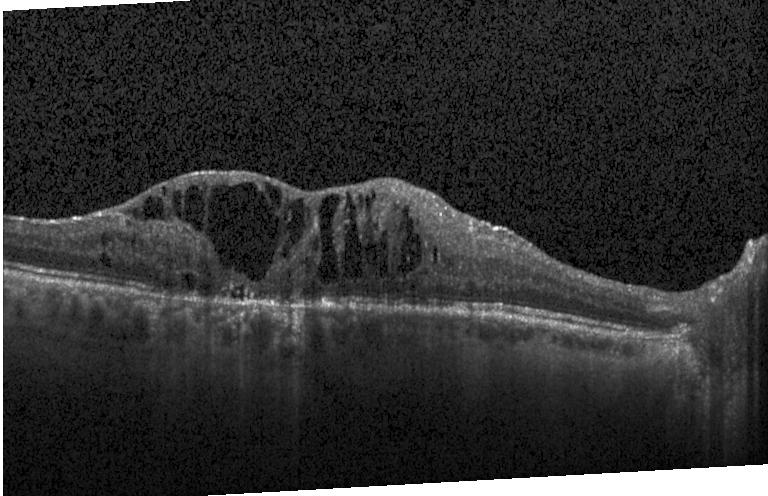 Diagnosis: diabetic macular edema (DME).